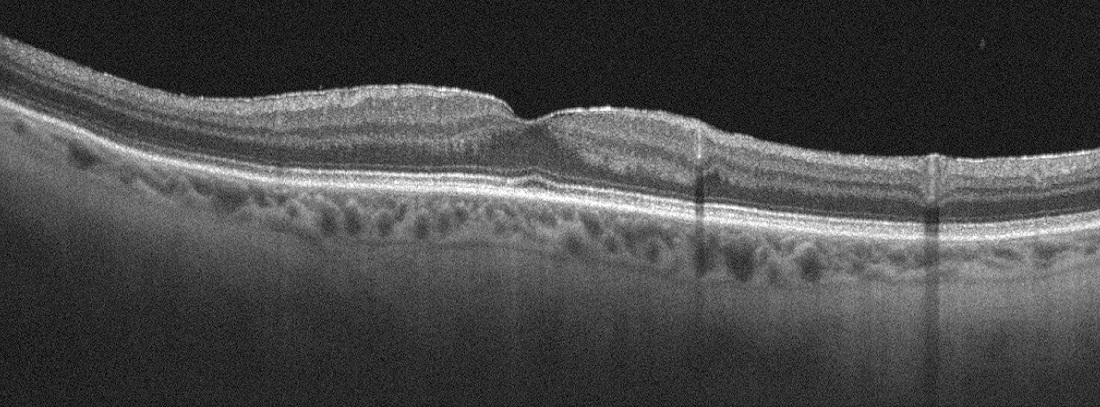 Epiretinal membrane (ERM).